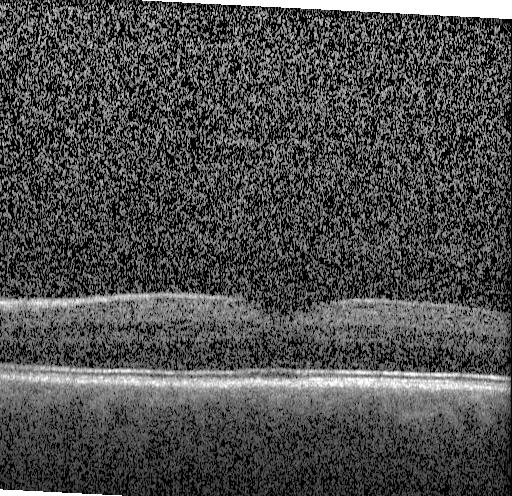 Impression: neither choroidal neovascularization, diabetic macular edema, nor drusen.